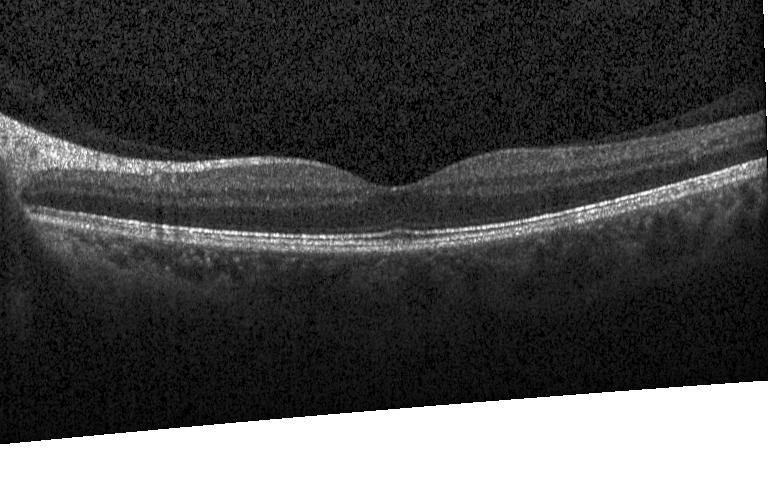

Dx: no choroidal neovascularization, no diabetic macular edema, and no drusen.